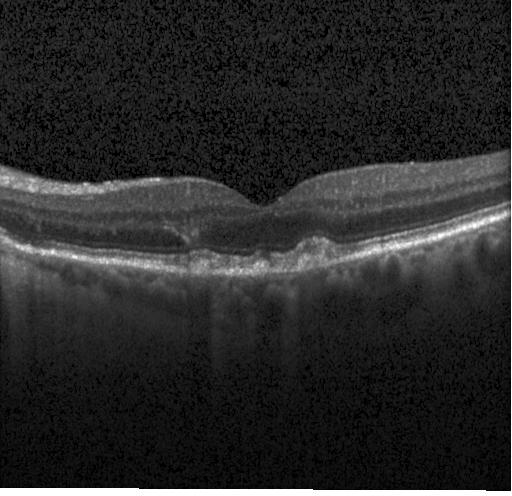

Macular scan · optical coherence tomography B-scan.
Impression: sub-RPE drusenoid deposits.